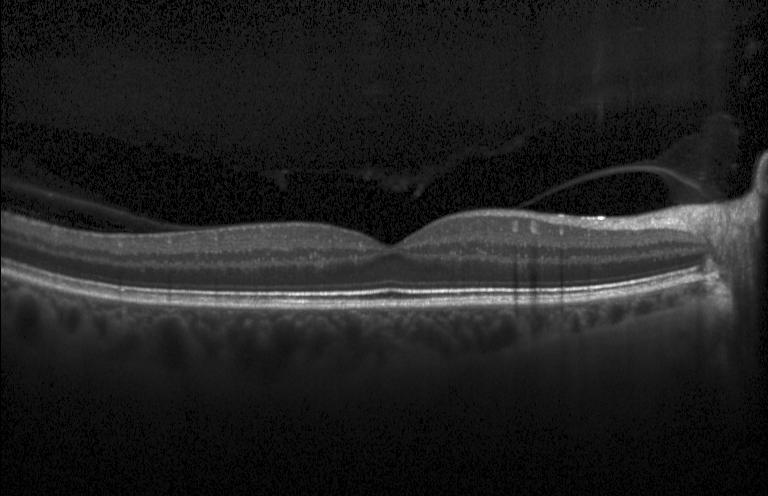
Instrument: Heidelberg Spectralis · retinal OCT cross-section.
Diagnosis: no CNV, DME, or drusen.